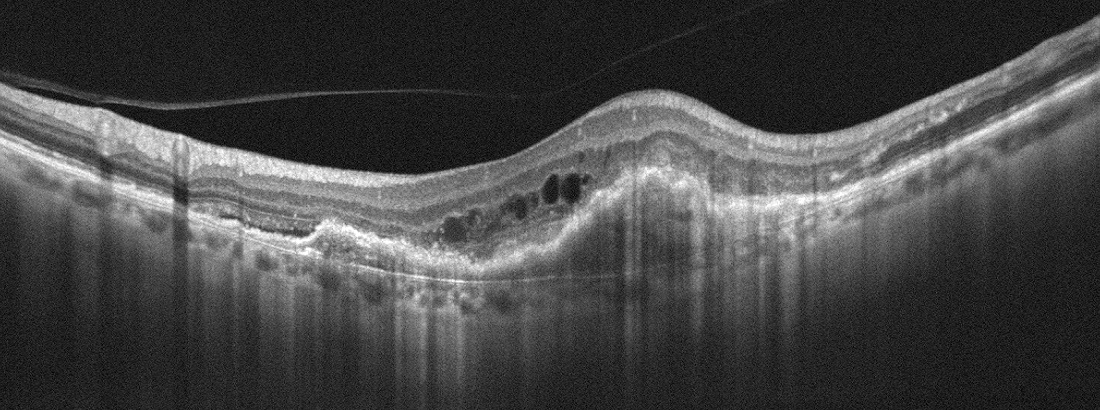 Impression: age-related macular degeneration.